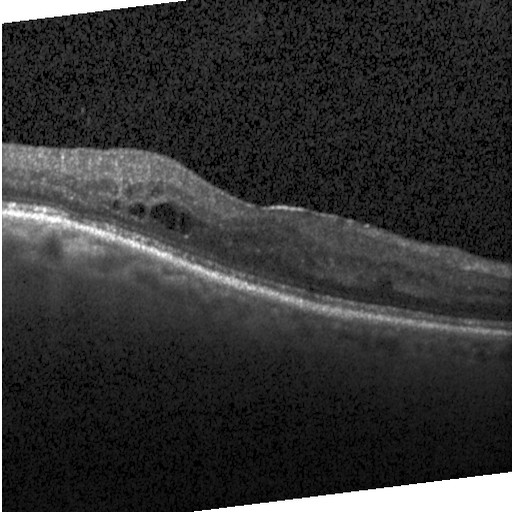 Spectral-domain optical coherence tomography; acquired on a Heidelberg Spectralis; fovea-centered; optical coherence tomography scan. The scan shows diabetic macular edema (DME).